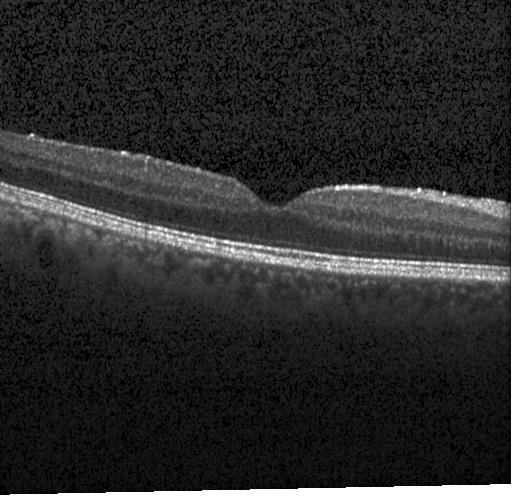
Diagnosis: neither choroidal neovascularization, diabetic macular edema, nor drusen.